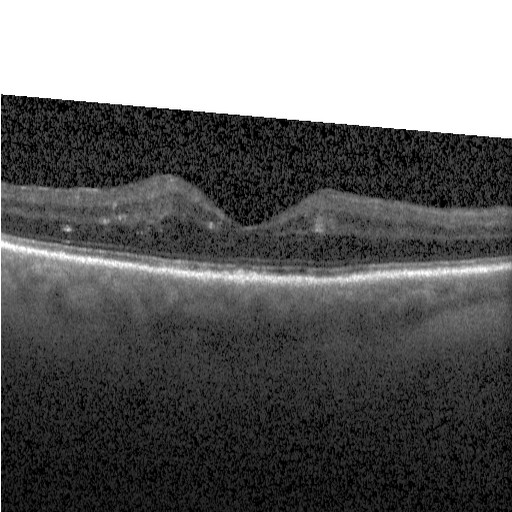

Through the macula, optical coherence tomography B-scan
Impression: diabetic macular edema (DME).